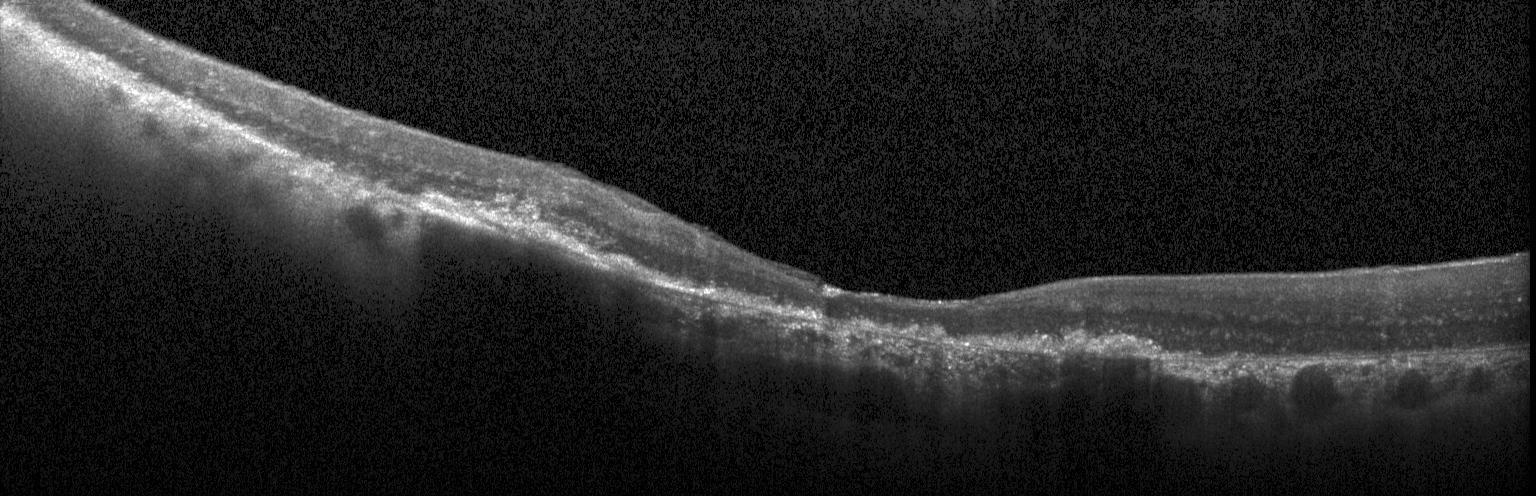
Fovea-centered · OCT line scan. Diagnosis: CNV.